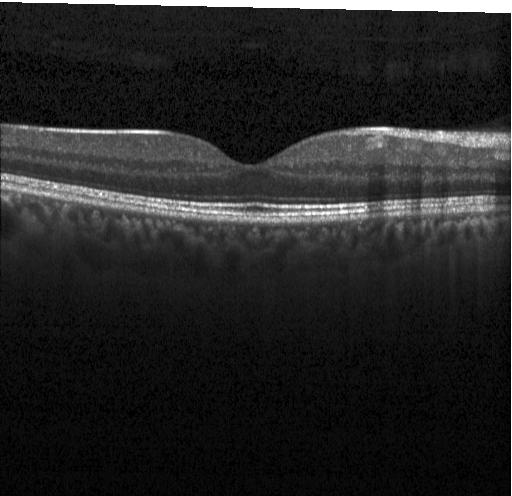
Spectral-domain optical coherence tomography, optical coherence tomography B-scan, centered on the fovea, acquired on a Heidelberg Spectralis.
Impression: no evidence of choroidal neovascularization, diabetic macular edema, or drusen.